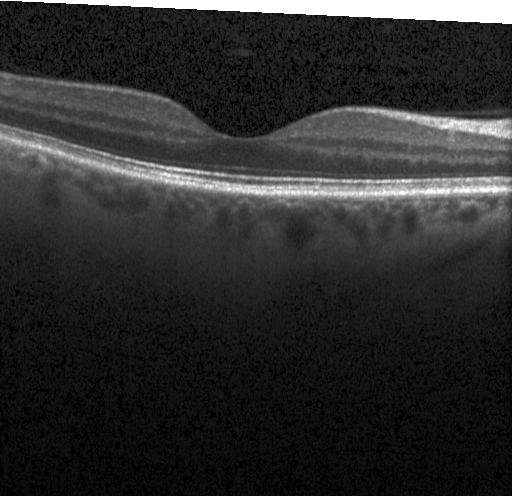 Acquired on a Heidelberg Spectralis · macular scan · SD-OCT · OCT line scan
This B-scan demonstrates neither CNV, DME, nor drusen.